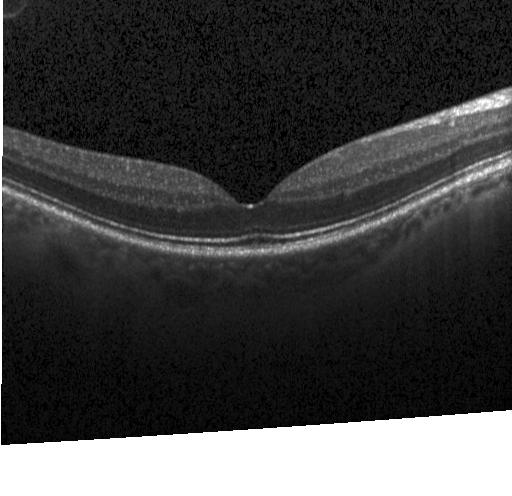 OCT line scan. Acquired on a Heidelberg Spectralis. Through the macula. Spectral-domain OCT. Diagnosis: no evidence of CNV, DME, or drusen.